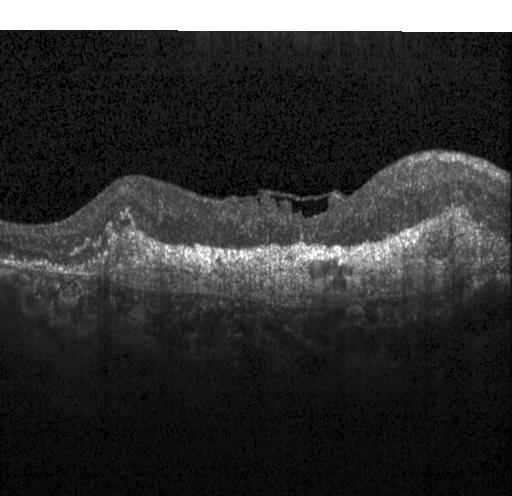 Retinal OCT B-scan. Spectral-domain optical coherence tomography. Acquired on a Heidelberg Spectralis — The scan shows choroidal neovascularization (CNV).